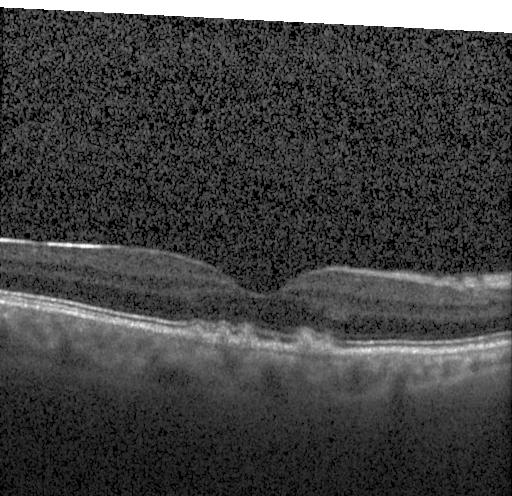

OCT scan showing drusen.